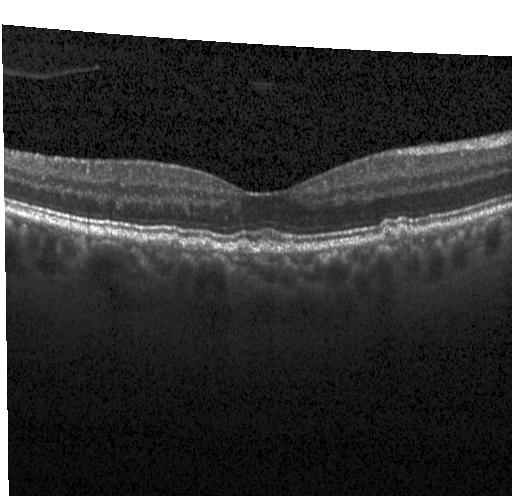 Through the macula. Spectral-domain optical coherence tomography. Optical coherence tomography B-scan — Finding: sub-RPE drusenoid deposits.